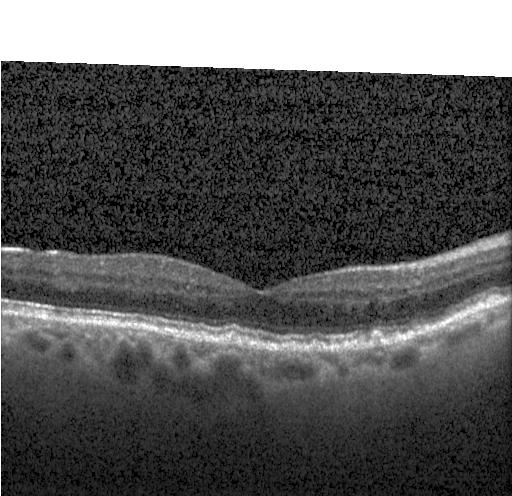

Impression: drusen.